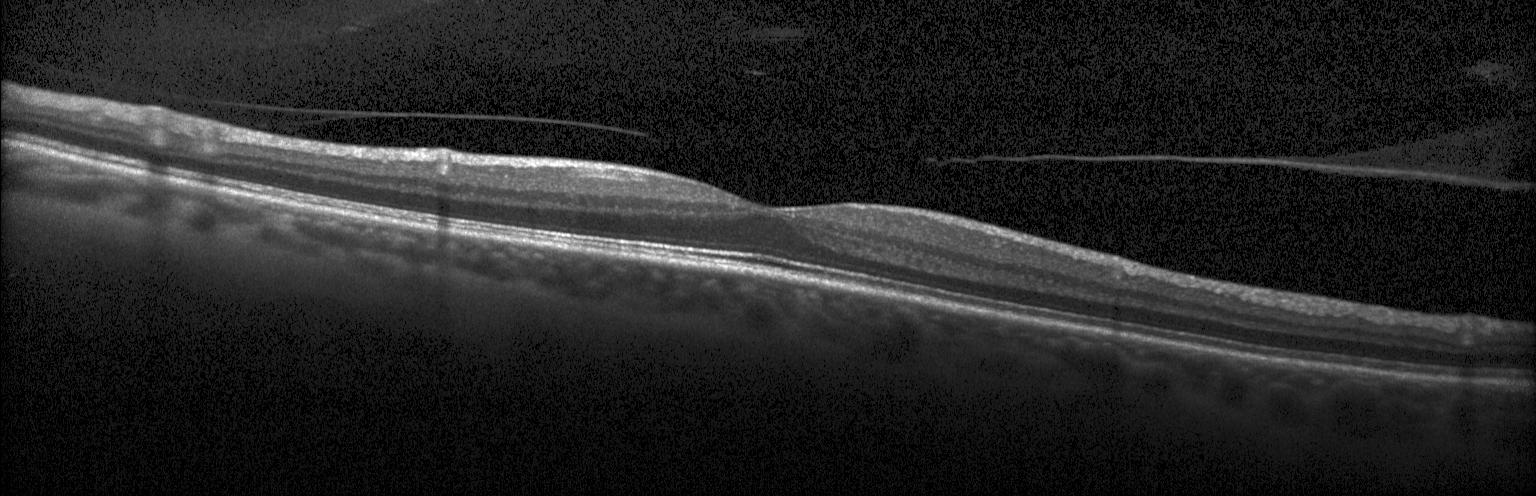

Diagnosis: no choroidal neovascularization, diabetic macular edema, or drusen.